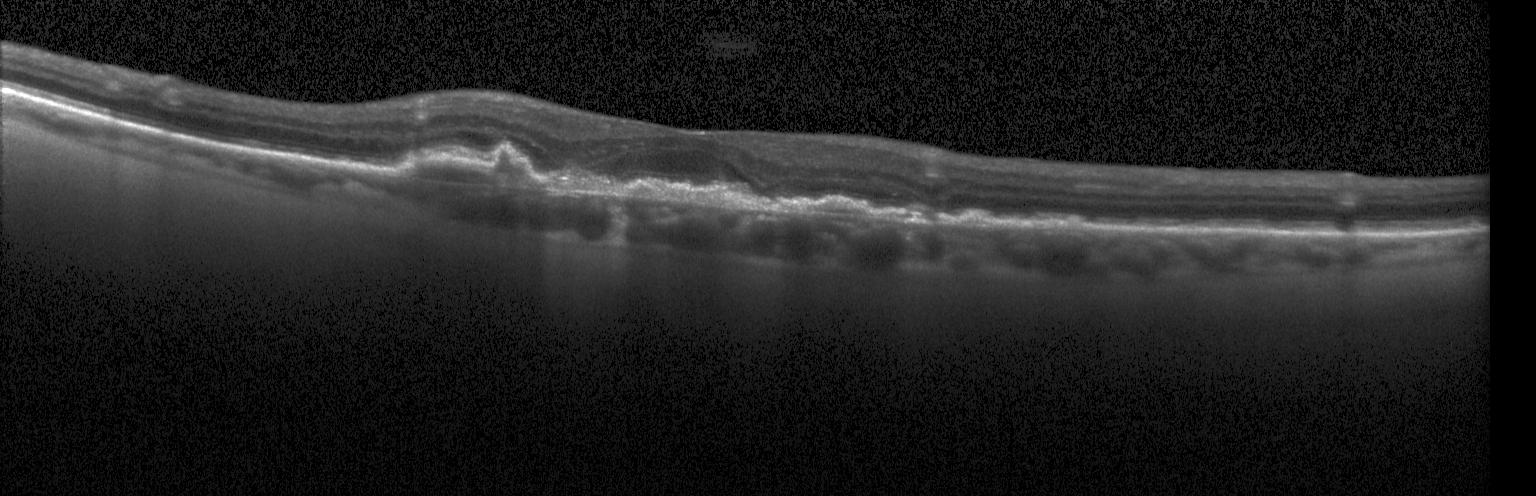
Spectral-domain OCT B-scan: a choroidal neovascular membrane.